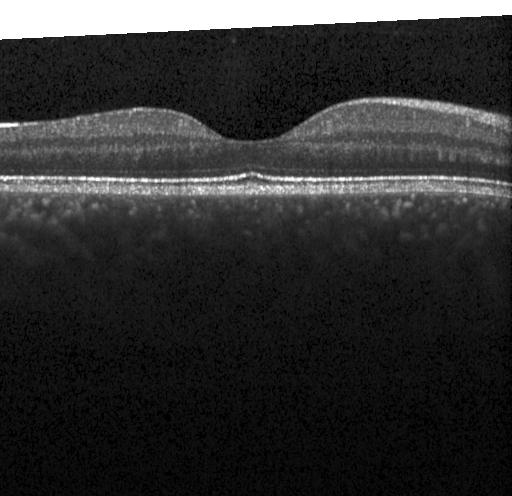

OCT B-scan. Spectral-domain optical coherence tomography
Assessment: no evidence of CNV, DME, or drusen.